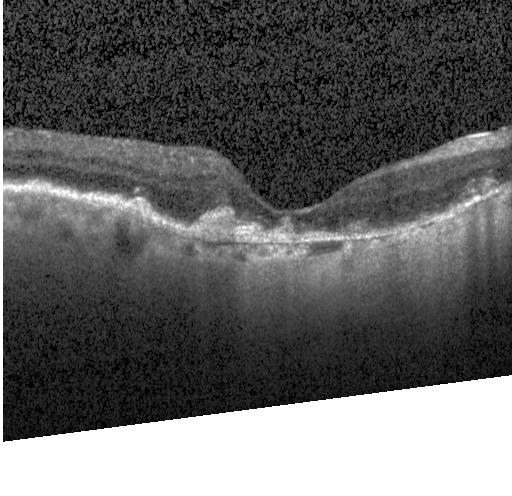
Retinal OCT cross-section showing a choroidal neovascular membrane.